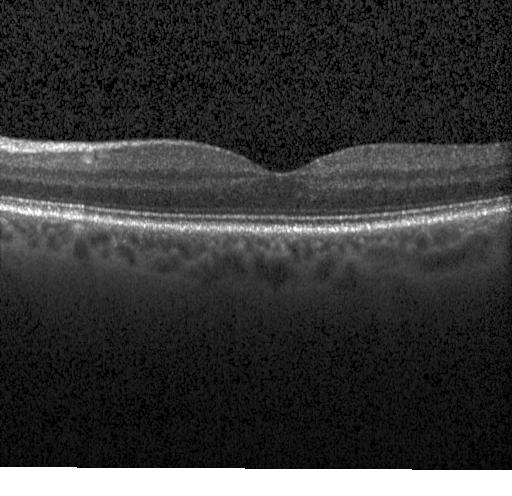
Macular scan; OCT line scan; instrument: Heidelberg Spectralis.
Impression: no CNV, no DME, and no drusen.